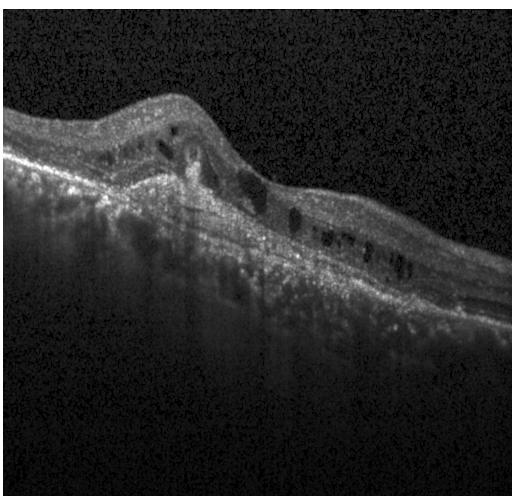

SD-OCT, optical coherence tomography scan, Heidelberg Spectralis.
Diagnosis: a choroidal neovascular membrane.